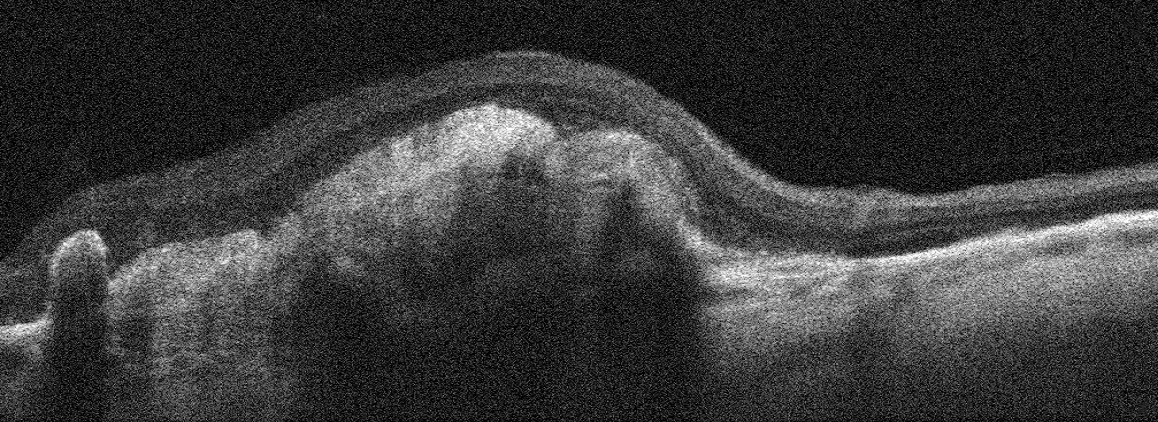

Right eye. Optical coherence tomography scan. Impression: AMD.